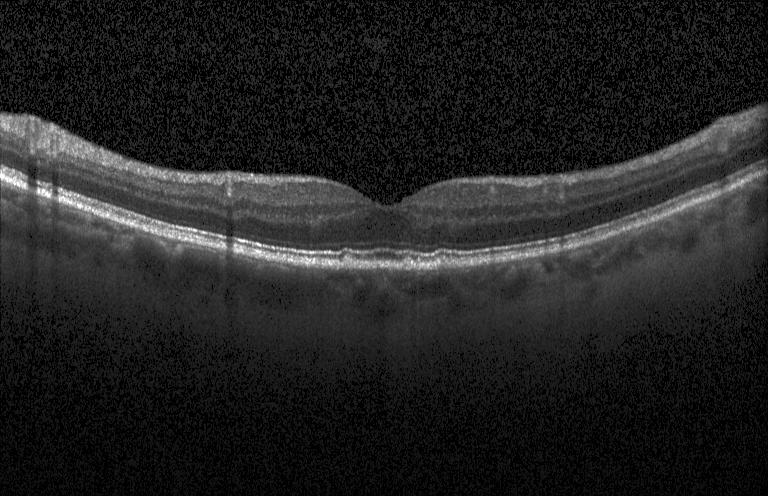 OCT scan showing sub-RPE drusenoid deposits.